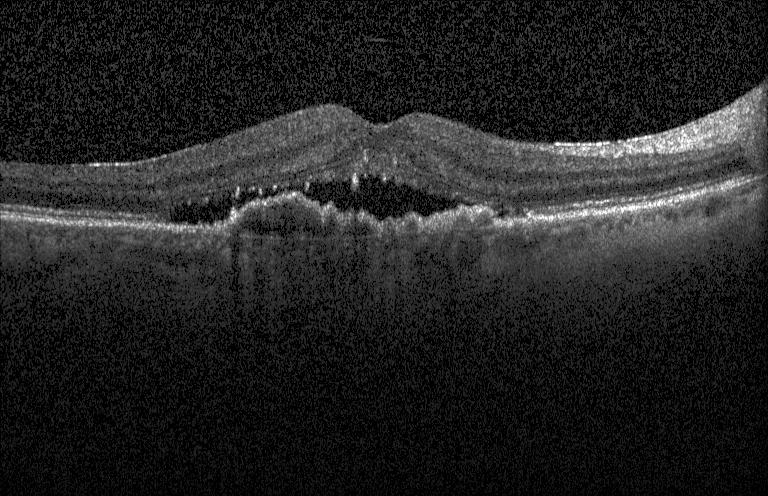

Retinal OCT B-scan; spectral-domain OCT; centered on the fovea; instrument: Heidelberg Spectralis — Impression: a choroidal neovascular membrane.